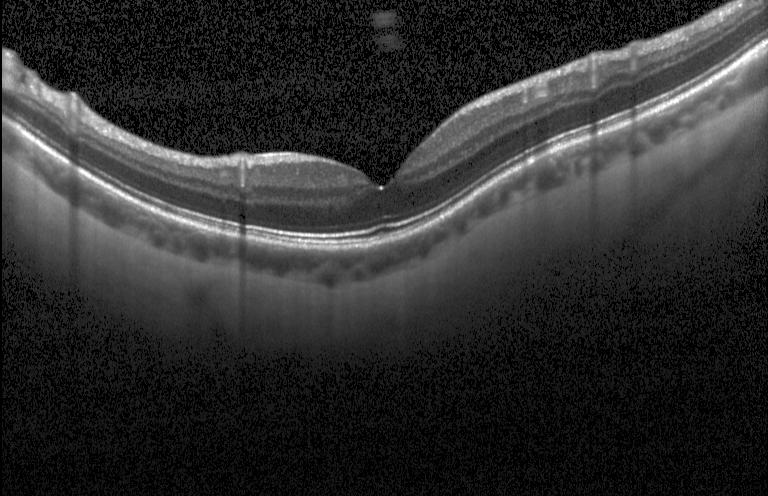
Finding: neither choroidal neovascularization, diabetic macular edema, nor drusen.